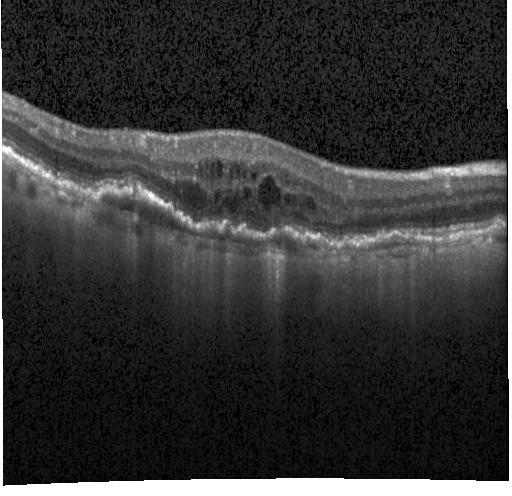
Instrument: Heidelberg Spectralis · retinal OCT cross-section — Macular OCT: choroidal neovascularization (CNV).